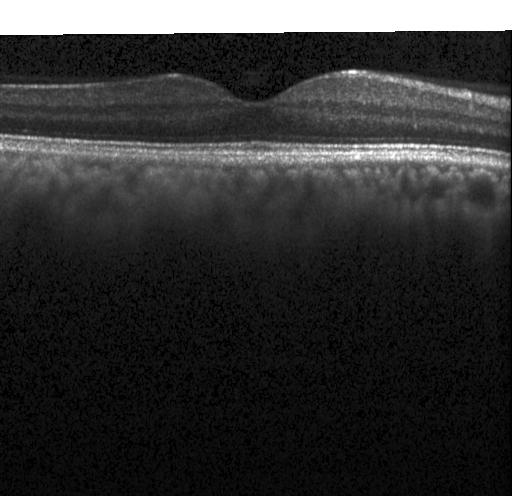

Retinal OCT B-scan, spectral-domain OCT, macular scan. OCT finding: neither choroidal neovascularization, diabetic macular edema, nor drusen.